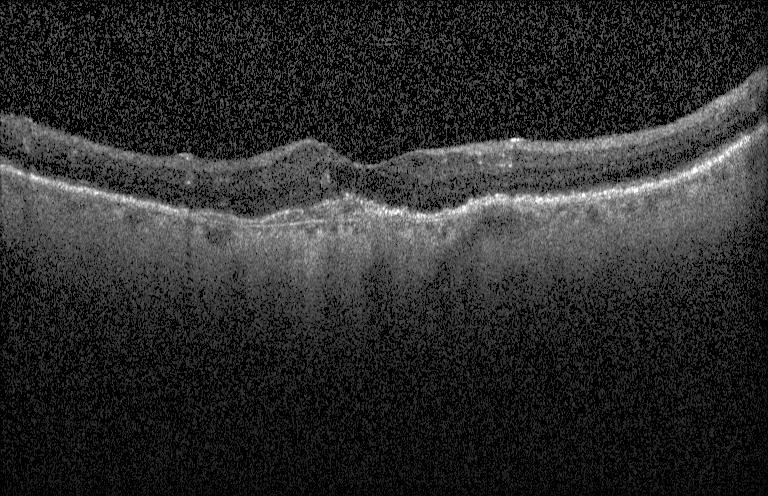
SD-OCT, OCT B-scan, instrument: Heidelberg Spectralis
Macular OCT: a choroidal neovascular membrane.